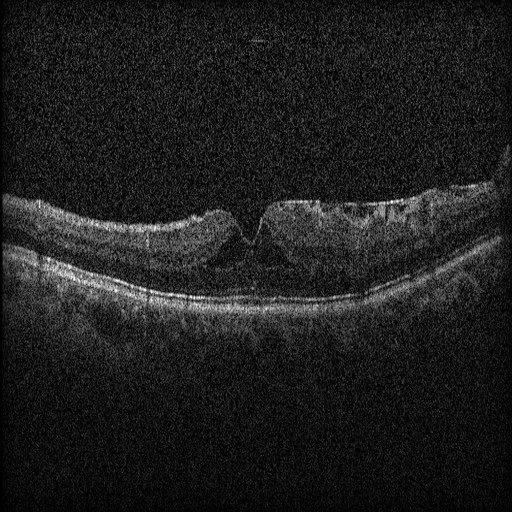
Horizontal scan through the fovea; Heidelberg Spectralis; OCT line scan — This B-scan demonstrates DME.